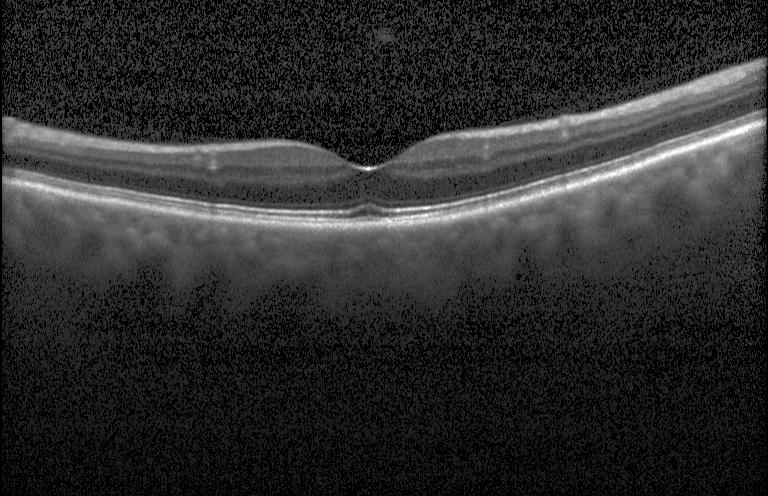
OCT B-scan showing no CNV, no DME, and no drusen.